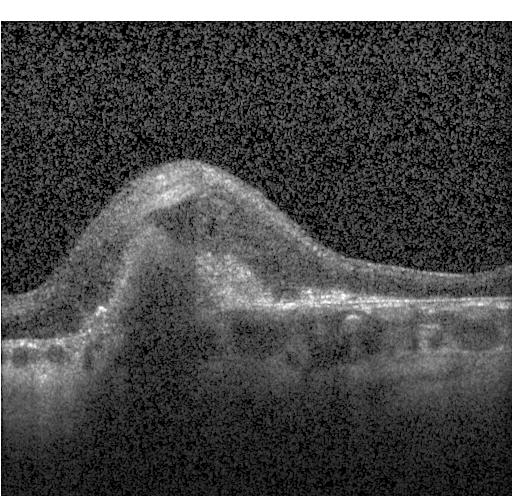
Centered on the fovea. OCT line scan. Finding: a choroidal neovascular membrane.